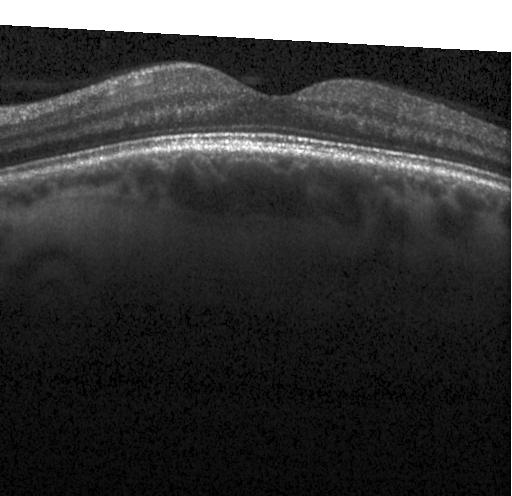

Spectral-domain OCT · acquired on a Heidelberg Spectralis · optical coherence tomography B-scan · fovea-centered.
Impression: neither choroidal neovascularization, diabetic macular edema, nor drusen.